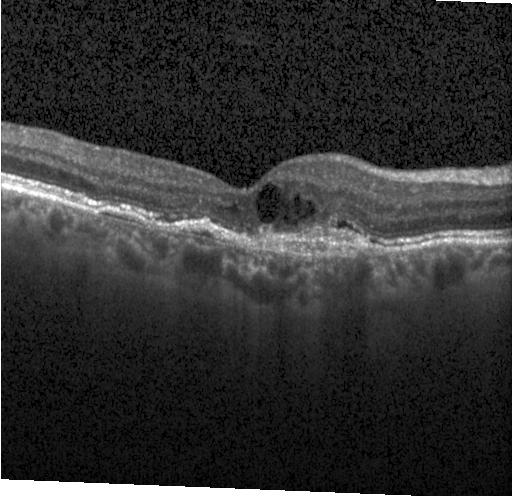 Retinal OCT B-scan, acquired on a Heidelberg Spectralis, centered on the fovea, spectral-domain optical coherence tomography.
A choroidal neovascular membrane.